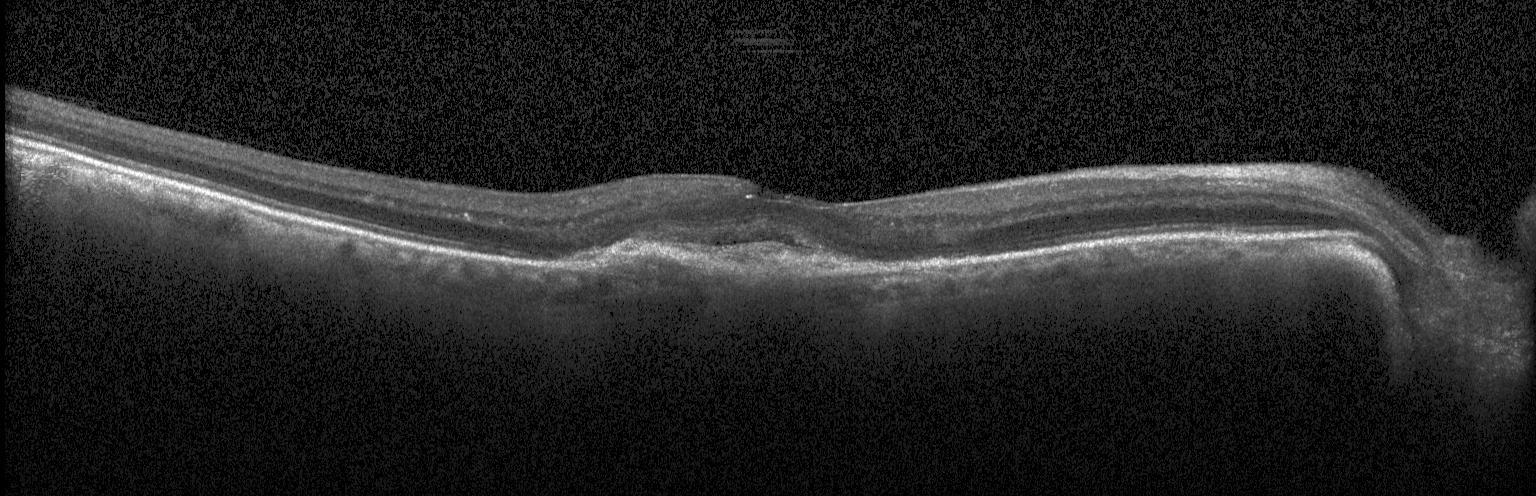

OCT line scan · Heidelberg Spectralis OCT system · SD-OCT · macular scan — Choroidal neovascularization (CNV).